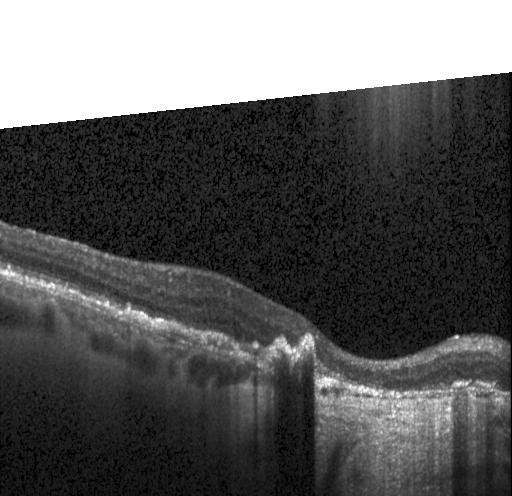
Acquired on a Heidelberg Spectralis · optical coherence tomography B-scan.
The scan shows a choroidal neovascular membrane.